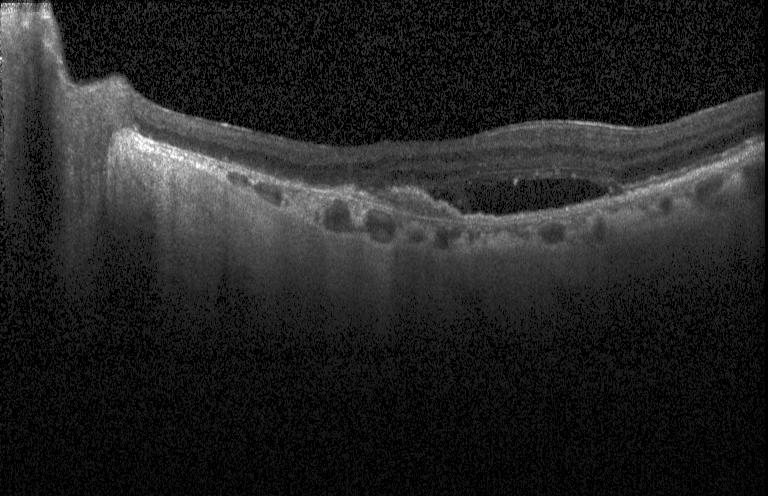

SD-OCT, OCT B-scan, Heidelberg Spectralis OCT system.
A choroidal neovascular membrane.